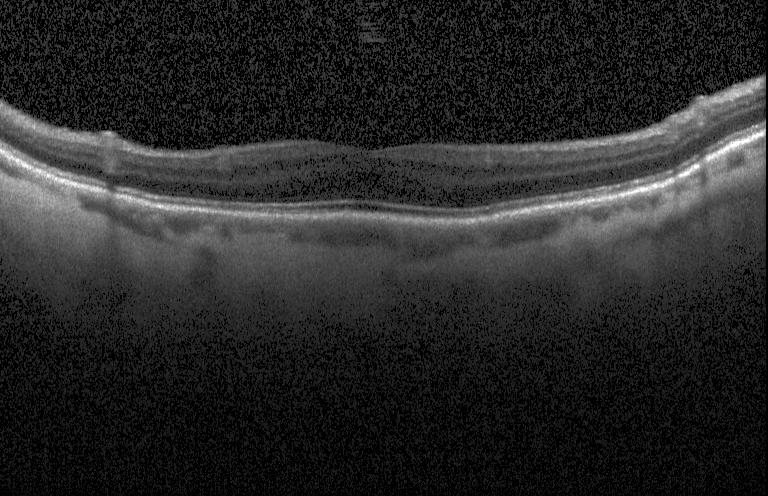

Acquired on a Heidelberg Spectralis · fovea-centered · spectral-domain optical coherence tomography · optical coherence tomography B-scan — The scan shows neither choroidal neovascularization, diabetic macular edema, nor drusen.